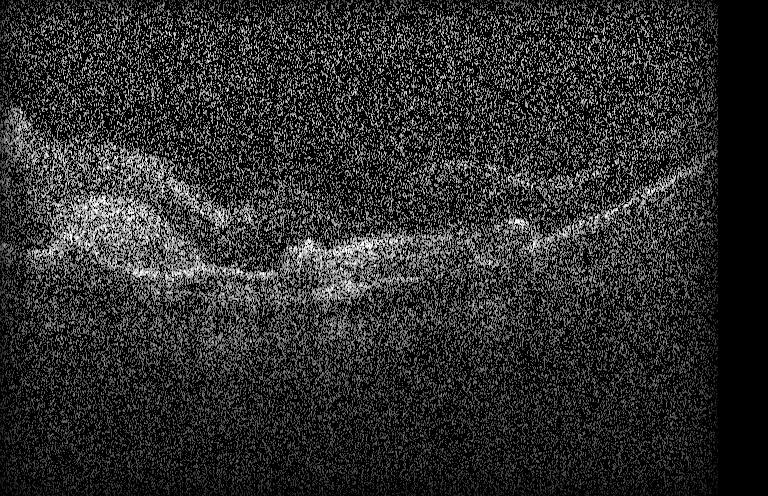

Spectral-domain OCT. Heidelberg Spectralis OCT system. Optical coherence tomography B-scan. Macular scan. This B-scan demonstrates choroidal neovascularization (CNV).